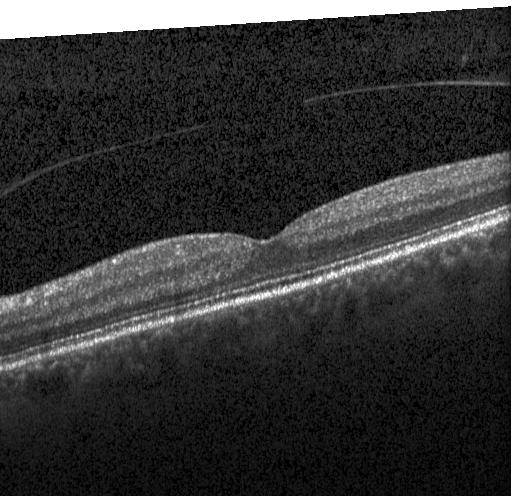
The scan shows no choroidal neovascularization, diabetic macular edema, or drusen.